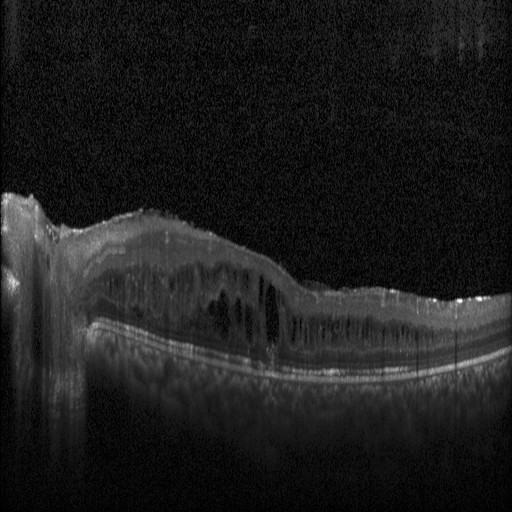 OCT B-scan.
Macular OCT: diabetic macular edema (DME).